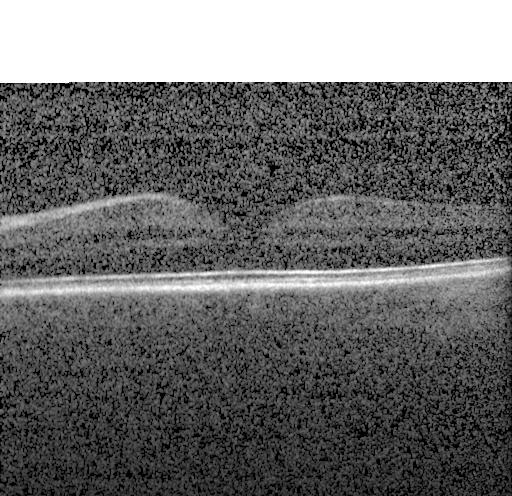 OCT B-scan — Assessment: no CNV, no DME, and no drusen.